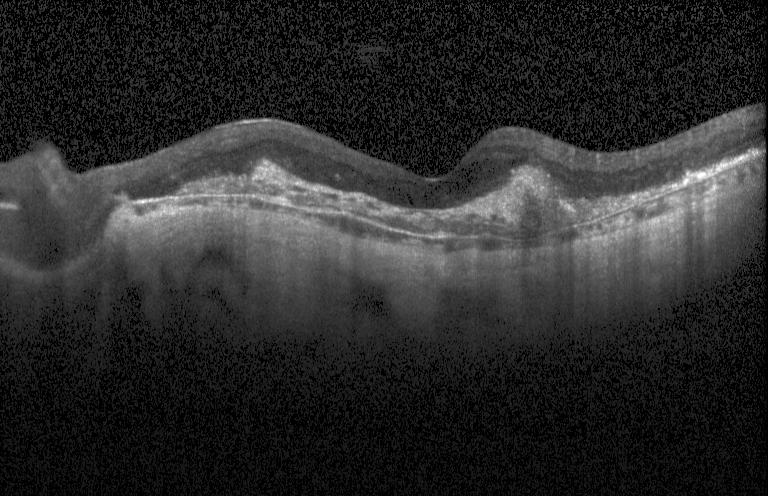 Finding: CNV.